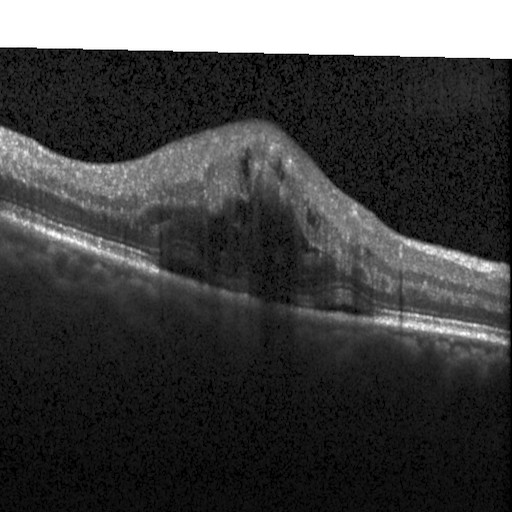 Instrument: Heidelberg Spectralis · spectral-domain OCT · horizontal scan through the fovea · optical coherence tomography B-scan — Impression: DME.